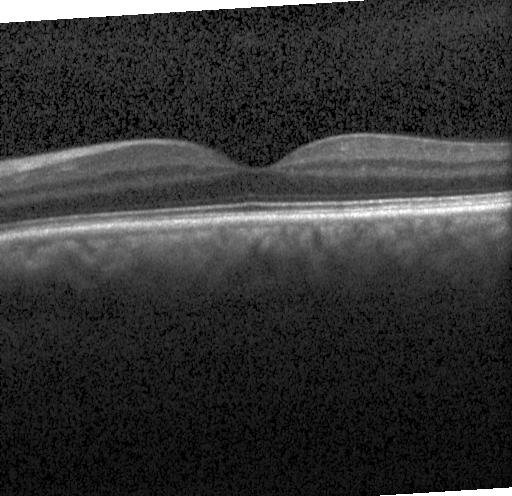 Impression: no CNV, DME, or drusen.